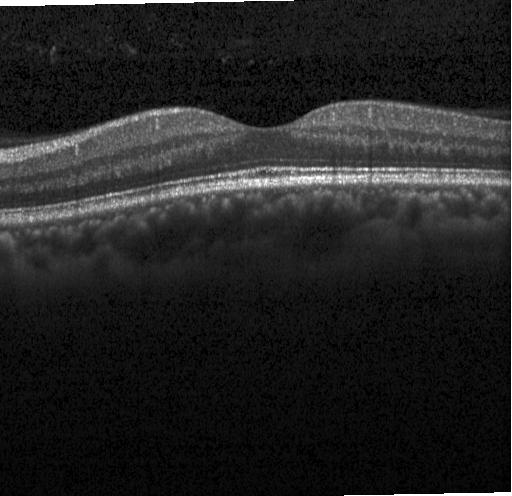
OCT B-scan · spectral-domain OCT.
This B-scan demonstrates no evidence of choroidal neovascularization, diabetic macular edema, or drusen.